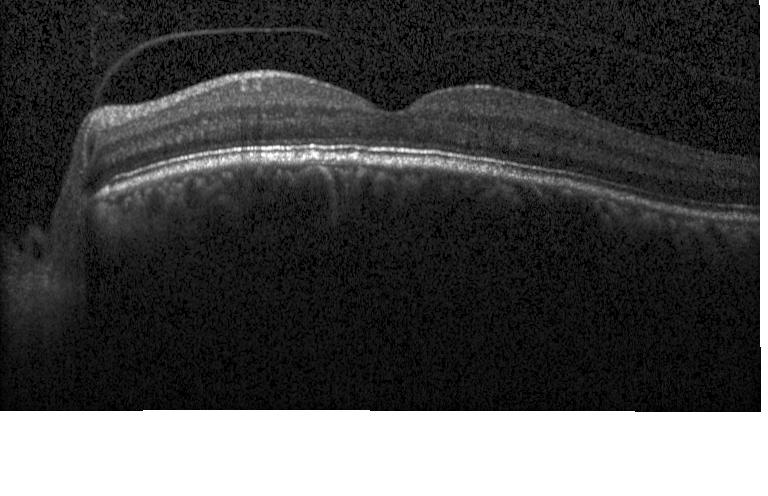
Retinal OCT cross-section — The scan shows neither CNV, DME, nor drusen.